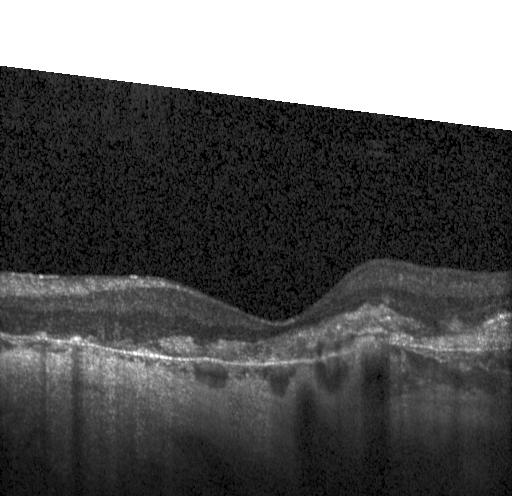 Optical coherence tomography B-scan.
This B-scan demonstrates a choroidal neovascular membrane.